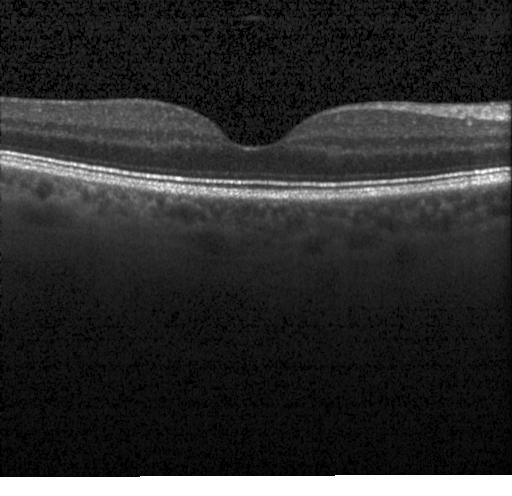

Macular OCT: no choroidal neovascularization, diabetic macular edema, or drusen.